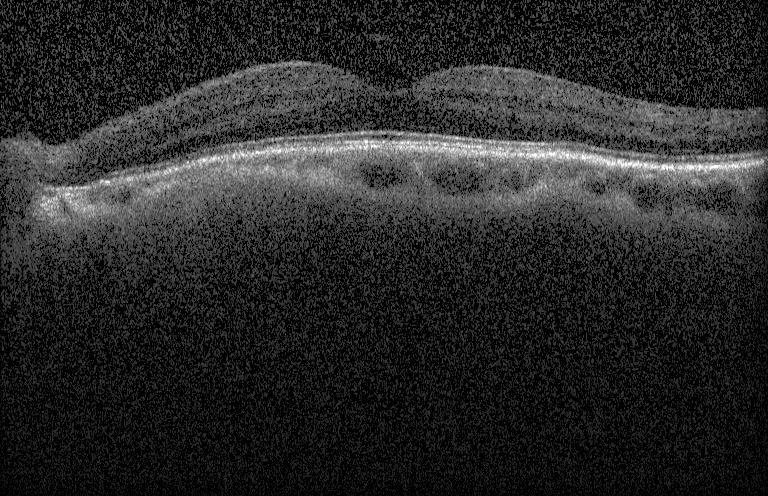 Impression: neither CNV, DME, nor drusen.